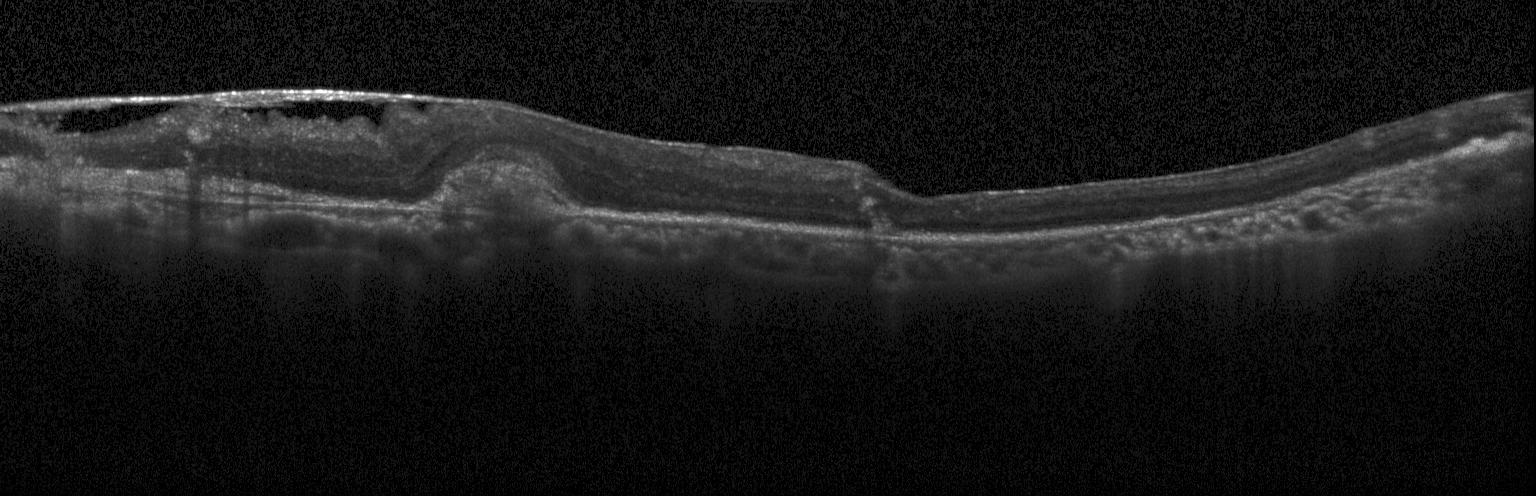

This B-scan demonstrates choroidal neovascularization (CNV).